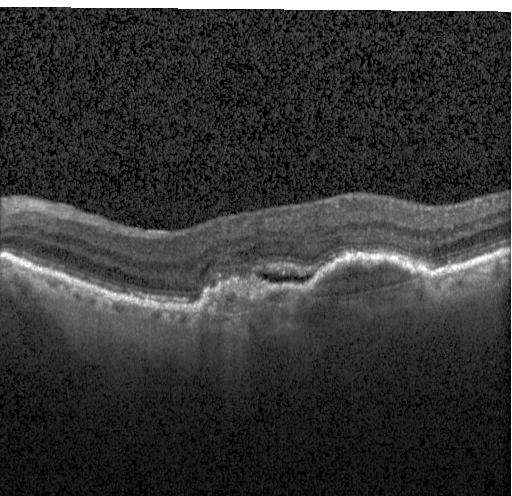 OCT line scan
OCT finding: a choroidal neovascular membrane.